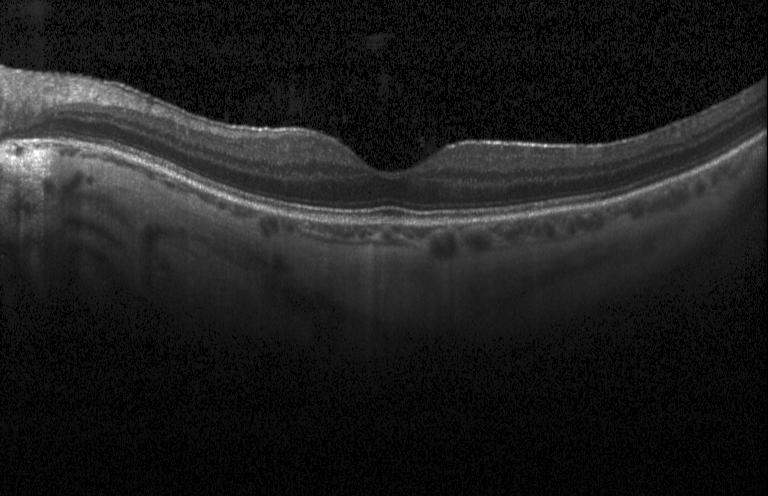
Macular OCT demonstrating no evidence of choroidal neovascularization, diabetic macular edema, or drusen.